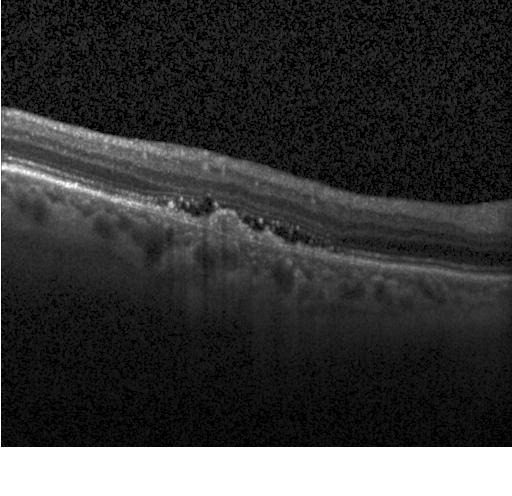
Impression: choroidal neovascularization.